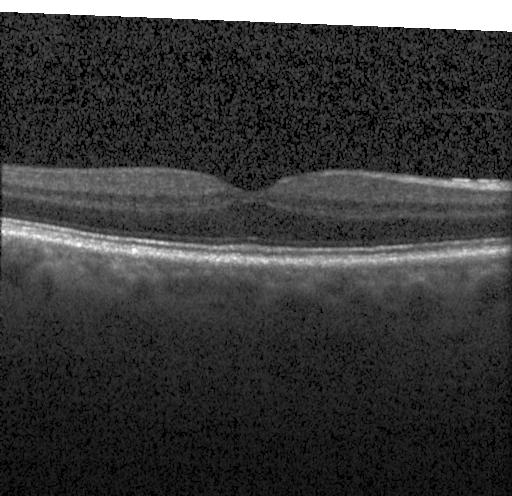

Instrument: Heidelberg Spectralis; optical coherence tomography B-scan; spectral-domain OCT.
Impression: neither CNV, DME, nor drusen.